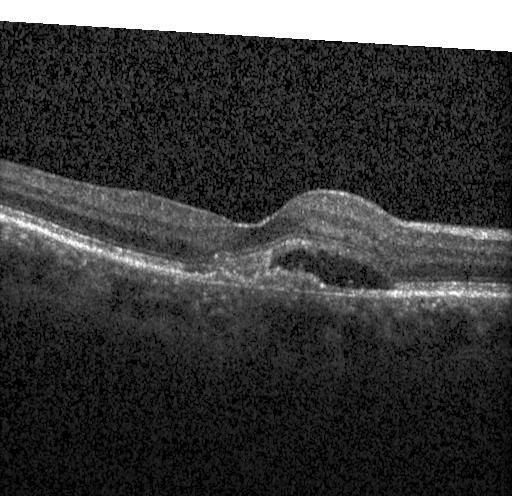

Macular scan, spectral-domain OCT, optical coherence tomography scan, acquired on a Heidelberg Spectralis.
Choroidal neovascularization (CNV).